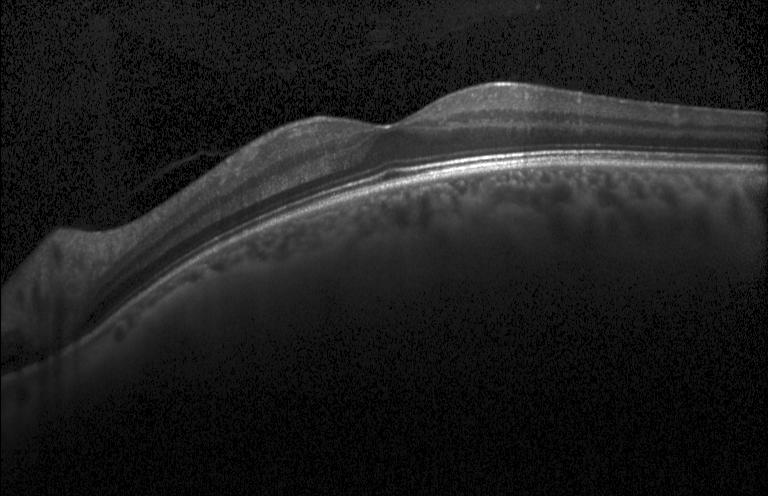

Spectral-domain OCT, optical coherence tomography scan, instrument: Heidelberg Spectralis.
No choroidal neovascularization, diabetic macular edema, or drusen.